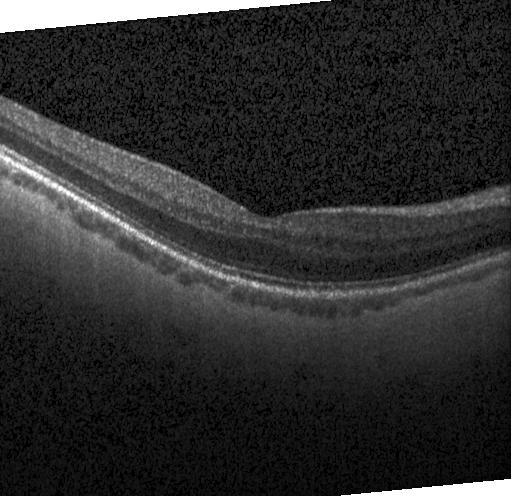
Optical coherence tomography B-scan; acquired on a Heidelberg Spectralis
Impression: no CNV, DME, or drusen.